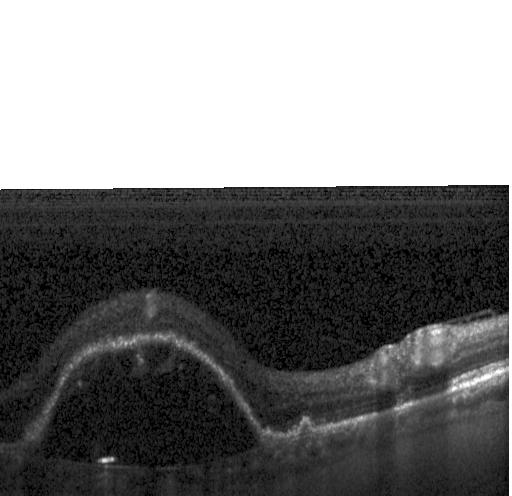 Retinal OCT cross-section · spectral-domain OCT — The scan shows CNV.